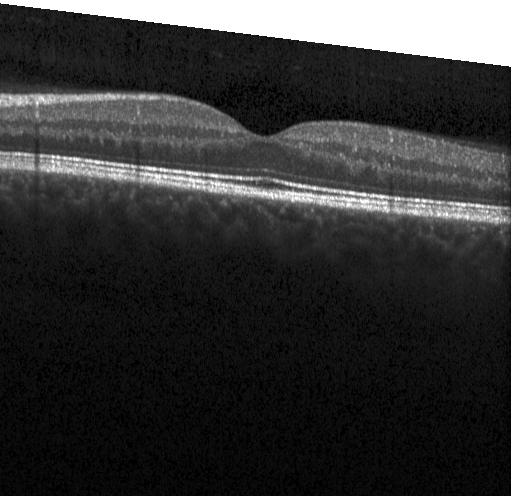

Instrument: Heidelberg Spectralis, through the macula, optical coherence tomography scan, spectral-domain optical coherence tomography — Diagnosis: neither choroidal neovascularization, diabetic macular edema, nor drusen.